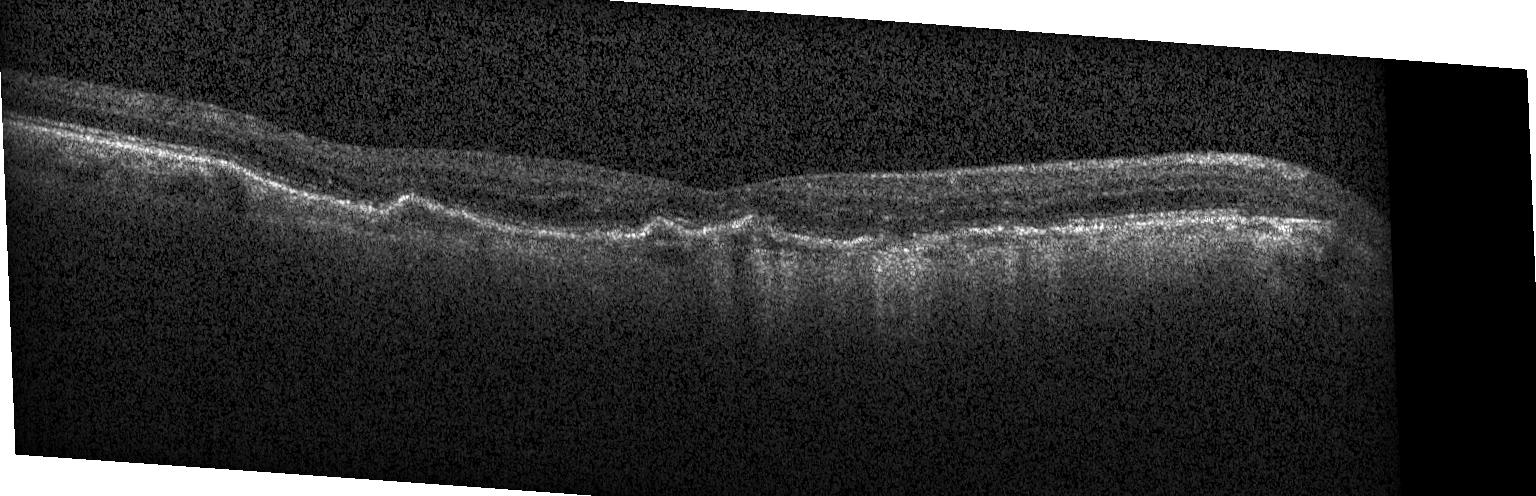 Macular OCT: choroidal neovascularization (CNV).